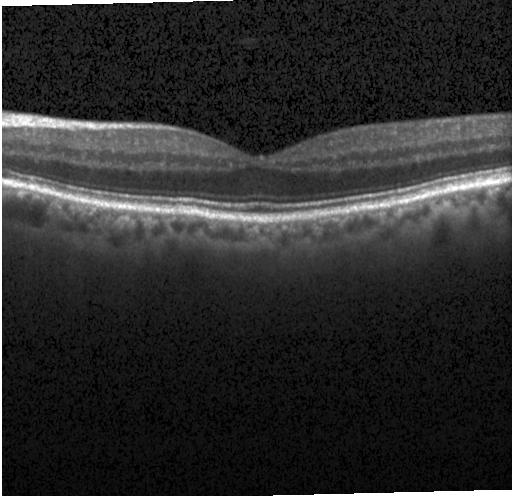

Neither CNV, DME, nor drusen.